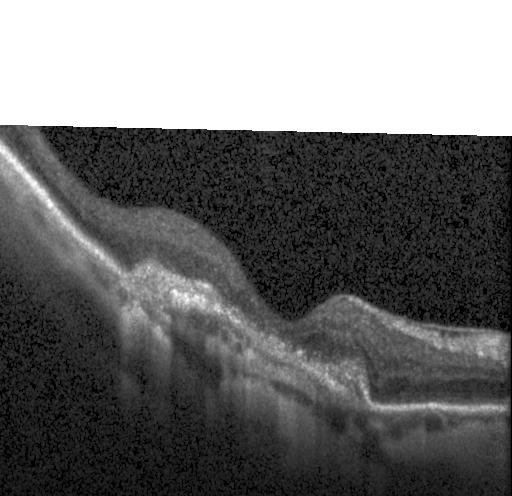

Optical coherence tomography scan. Heidelberg Spectralis OCT system
Diagnosis: choroidal neovascularization (CNV).